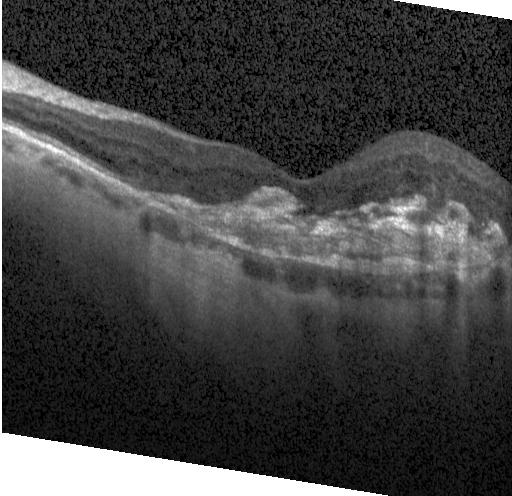
SD-OCT, OCT line scan — The scan shows choroidal neovascularization.